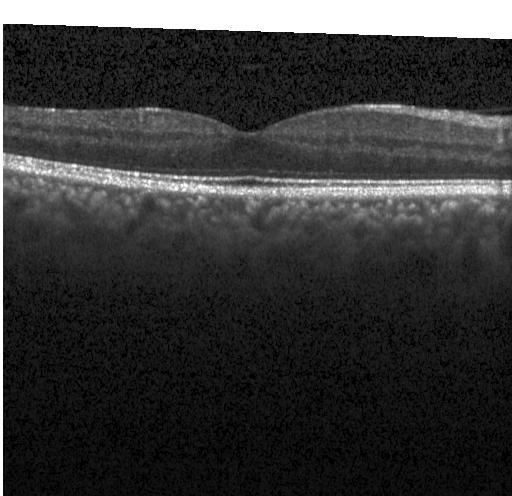 OCT line scan; macular scan; Heidelberg Spectralis. Macular OCT: neither choroidal neovascularization, diabetic macular edema, nor drusen.